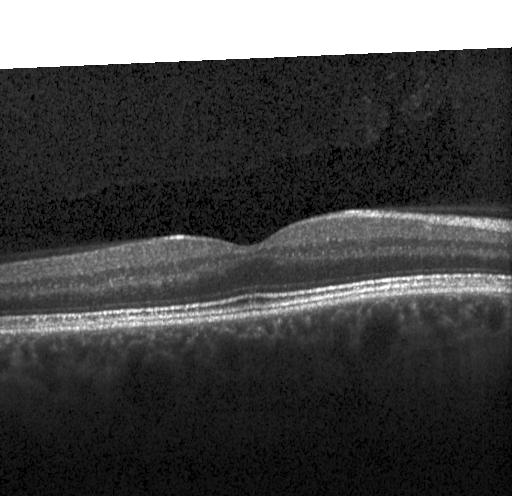 OCT B-scan showing neither choroidal neovascularization, diabetic macular edema, nor drusen.